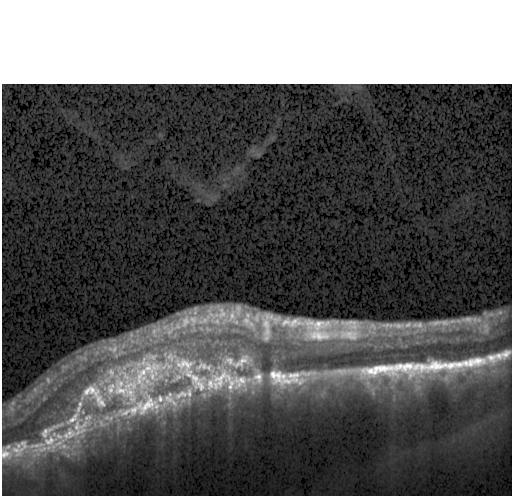

Through the macula. OCT B-scan. SD-OCT. Impression: a choroidal neovascular membrane.